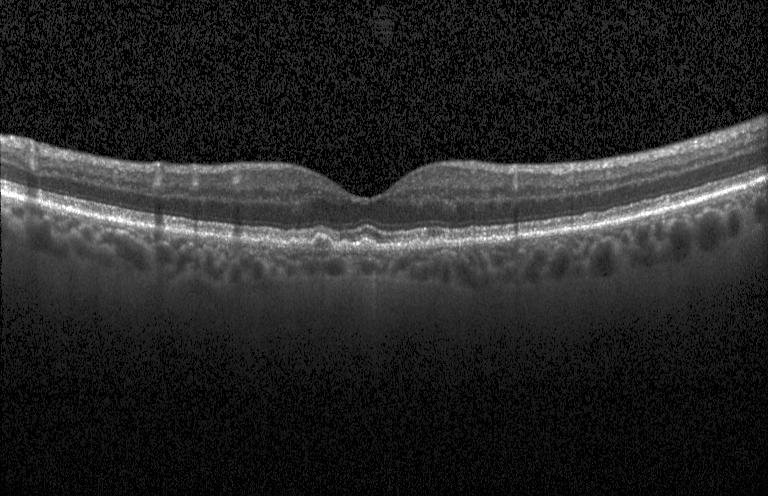 Optical coherence tomography B-scan
Drusen.